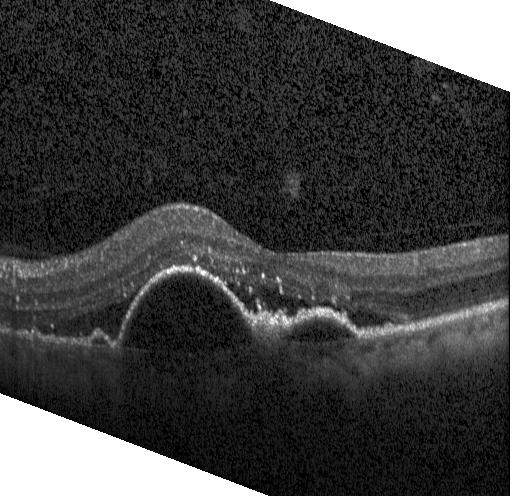

The scan shows a choroidal neovascular membrane.